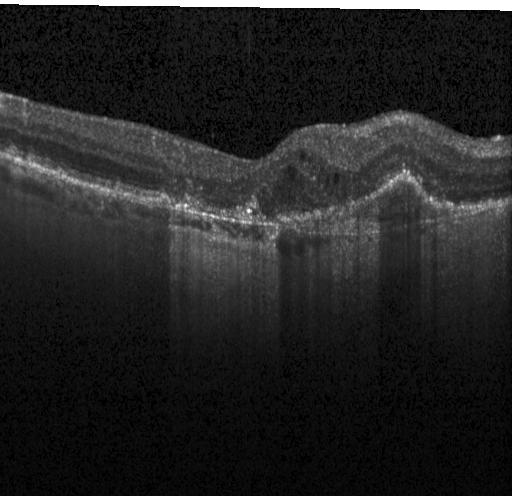 Retinal OCT cross-section showing a choroidal neovascular membrane.